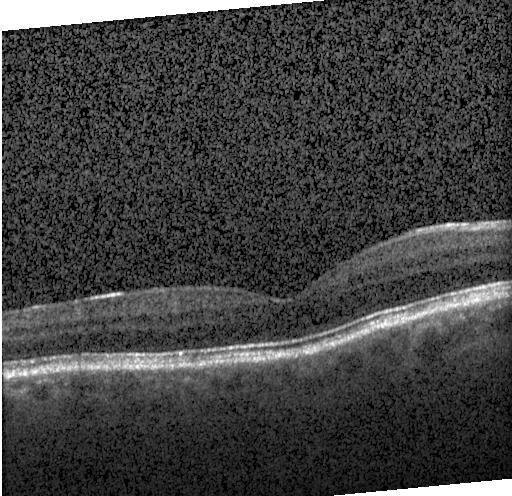 Heidelberg Spectralis OCT system. SD-OCT. Optical coherence tomography scan.
Finding: no choroidal neovascularization, no diabetic macular edema, and no drusen.